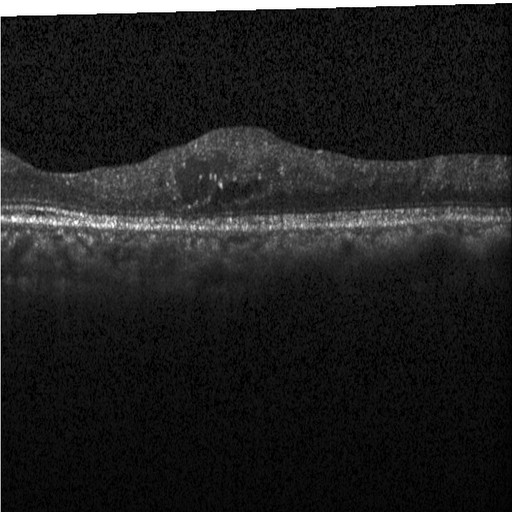

Retinal OCT cross-section showing diabetic macular edema.